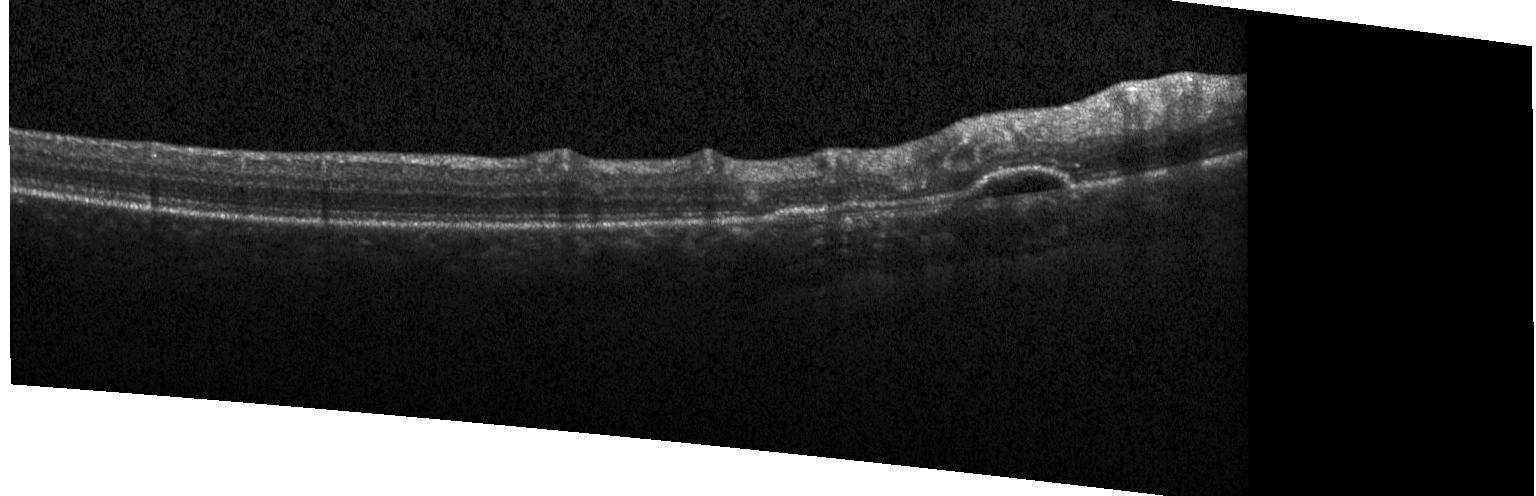

OCT B-scan; macular scan.
Impression: a choroidal neovascular membrane.